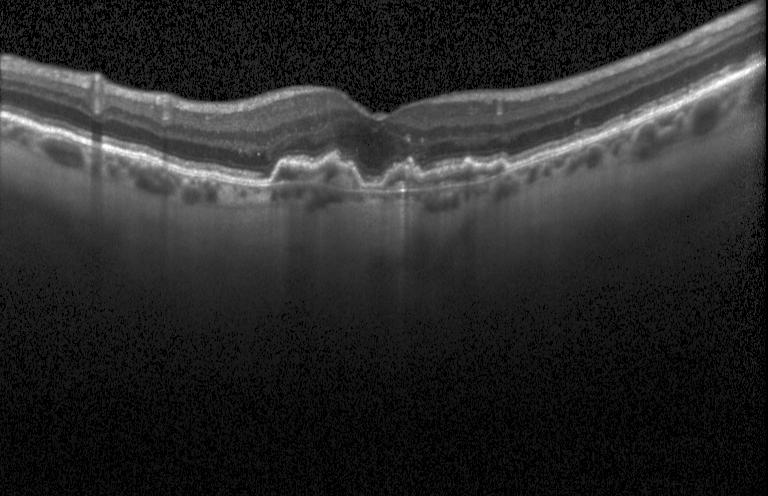
Spectral-domain OCT, horizontal scan through the fovea, retinal OCT B-scan.
Choroidal neovascularization (CNV).